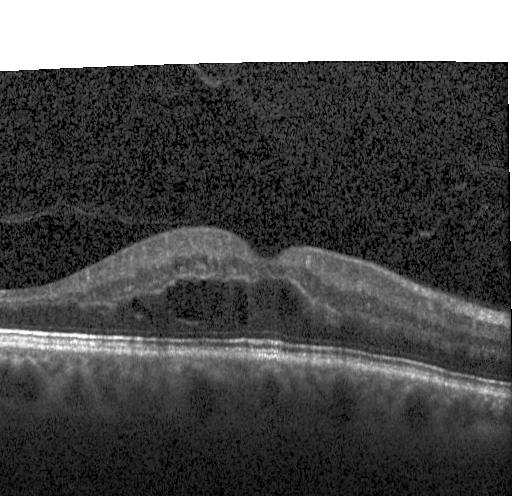
Retinal OCT cross-section · fovea-centered — Diagnosis: diabetic macular edema (DME).